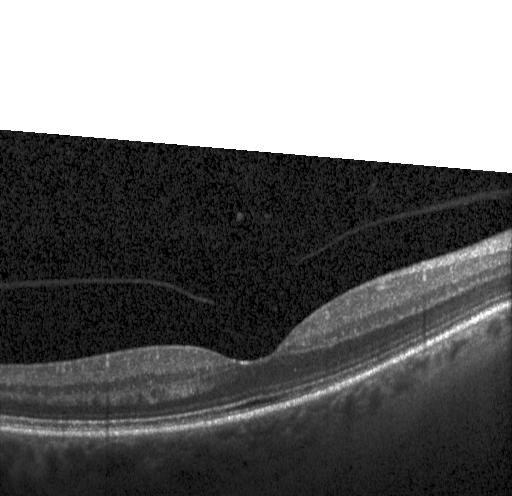

SD-OCT, OCT B-scan. This B-scan demonstrates no CNV, no DME, and no drusen.